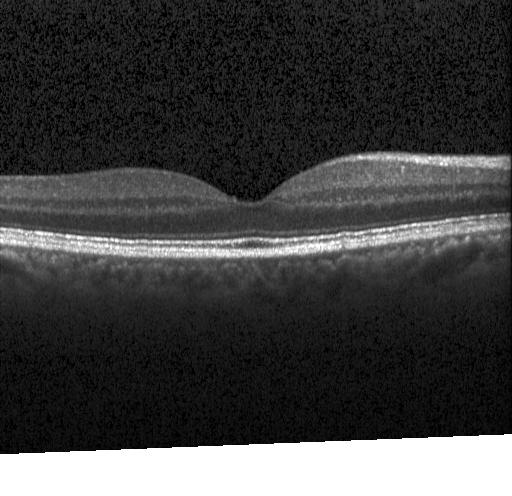 Impression: neither choroidal neovascularization, diabetic macular edema, nor drusen.